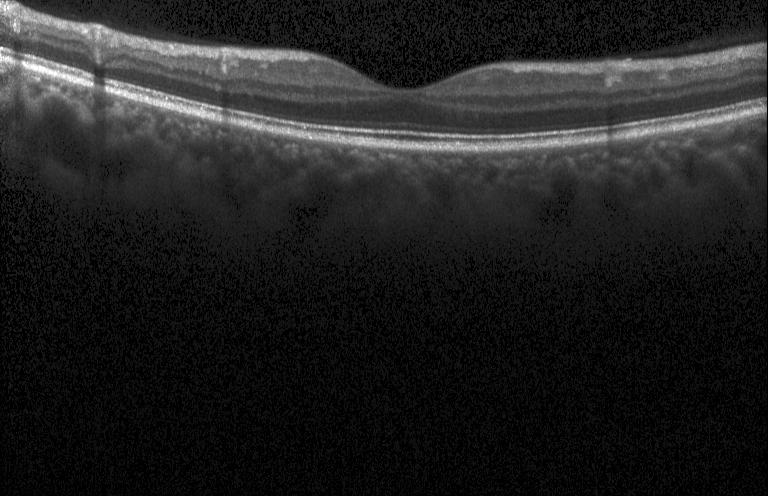 Assessment: no evidence of choroidal neovascularization, diabetic macular edema, or drusen.